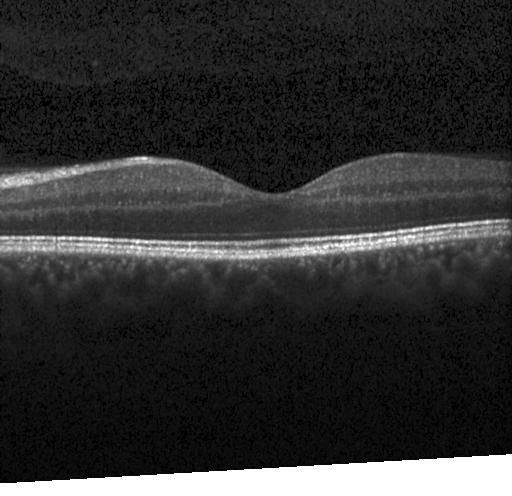

OCT B-scan showing no evidence of choroidal neovascularization, diabetic macular edema, or drusen.